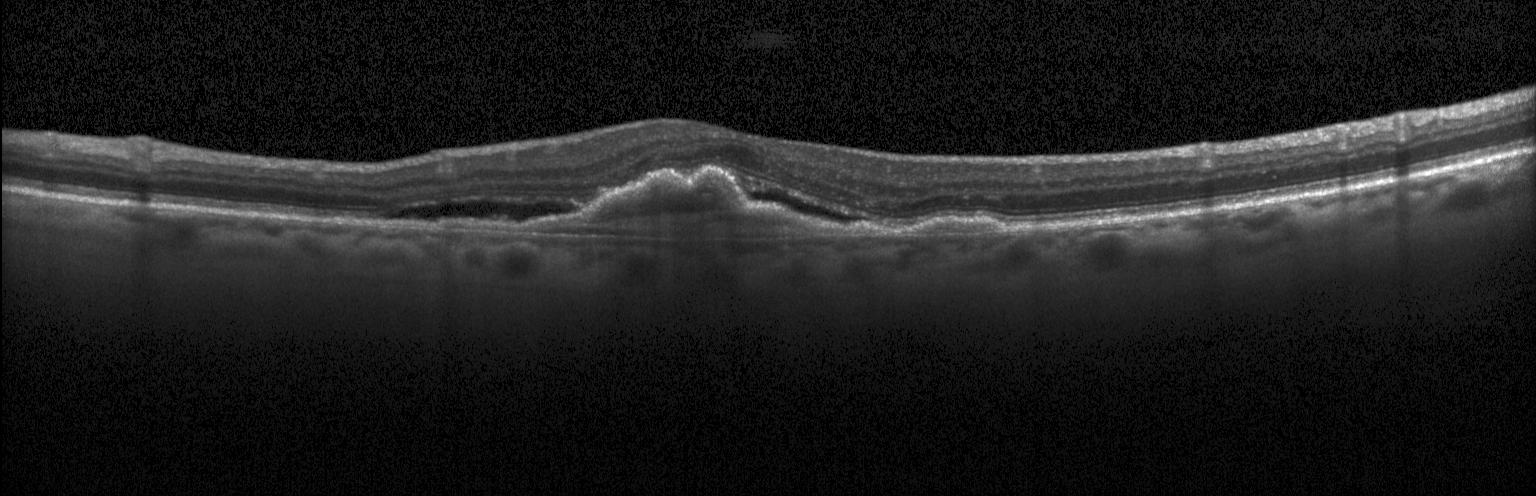

Optical coherence tomography B-scan · acquired on a Heidelberg Spectralis · SD-OCT · macular scan — Impression: CNV.